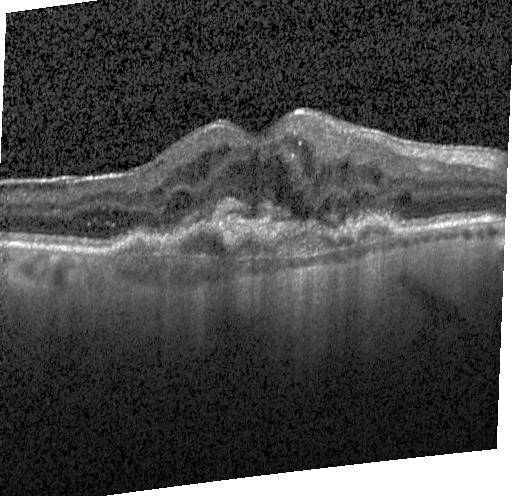

Optical coherence tomography scan. Diagnosis: a choroidal neovascular membrane.